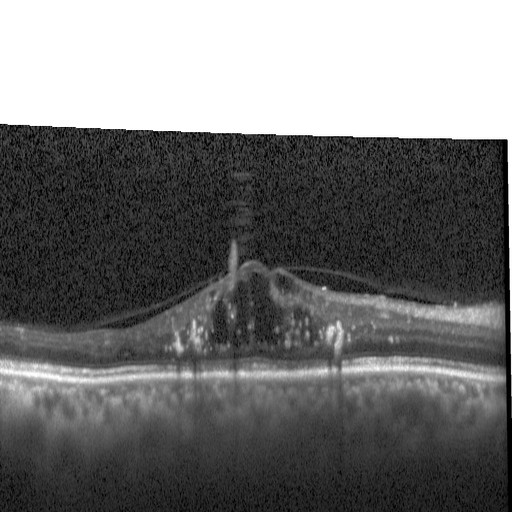

Diabetic macular edema (DME).